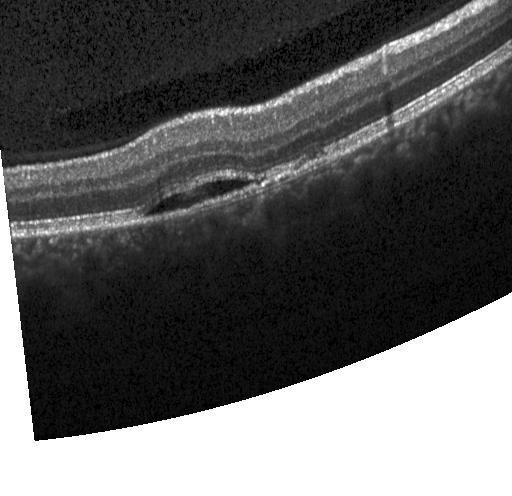
Horizontal scan through the fovea; OCT line scan. Finding: a choroidal neovascular membrane.